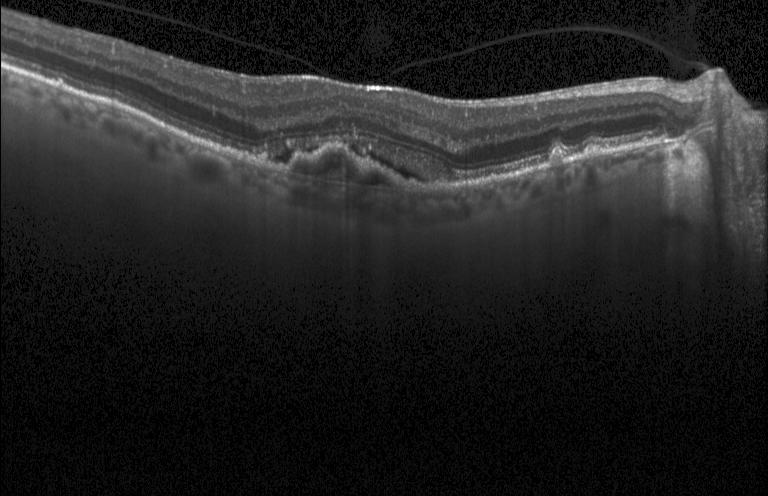

Fovea-centered · spectral-domain OCT · acquired on a Heidelberg Spectralis · optical coherence tomography scan — Diagnosis: a choroidal neovascular membrane.